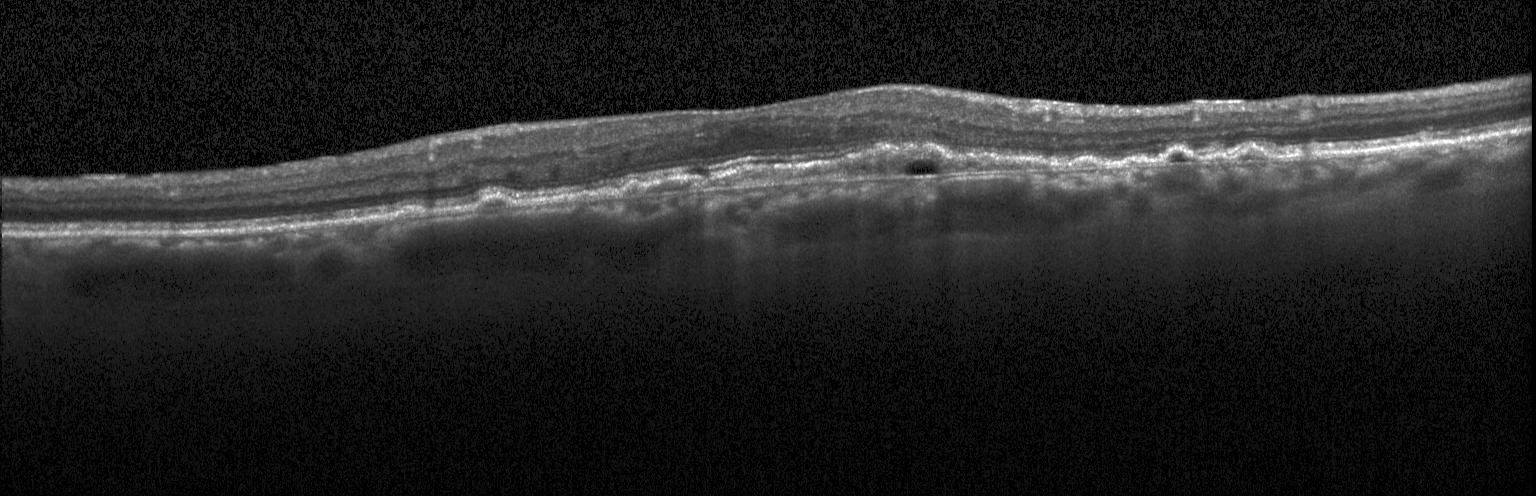 OCT B-scan
The scan shows choroidal neovascularization.